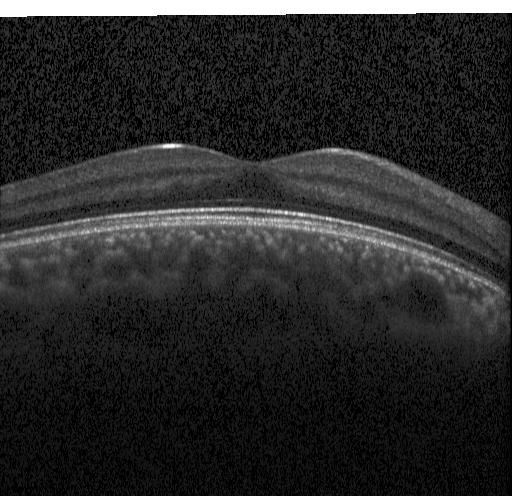

Retinal OCT cross-section; spectral-domain optical coherence tomography; fovea-centered
Diagnosis: no choroidal neovascularization, no diabetic macular edema, and no drusen.